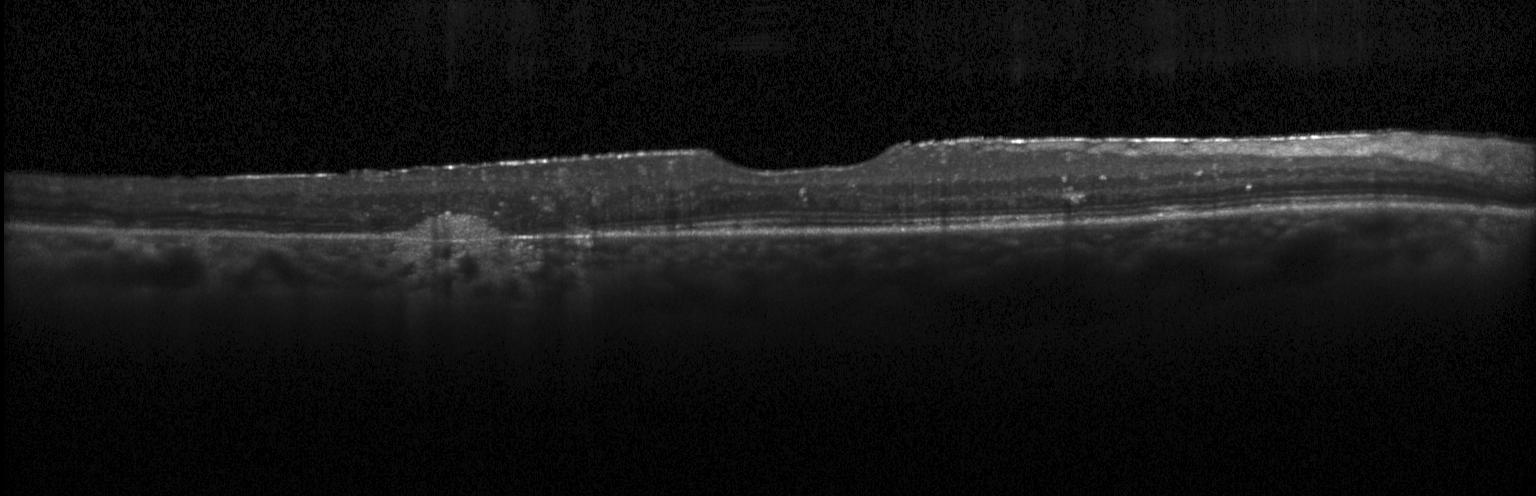
Centered on the fovea, optical coherence tomography B-scan, SD-OCT — This B-scan demonstrates a choroidal neovascular membrane.